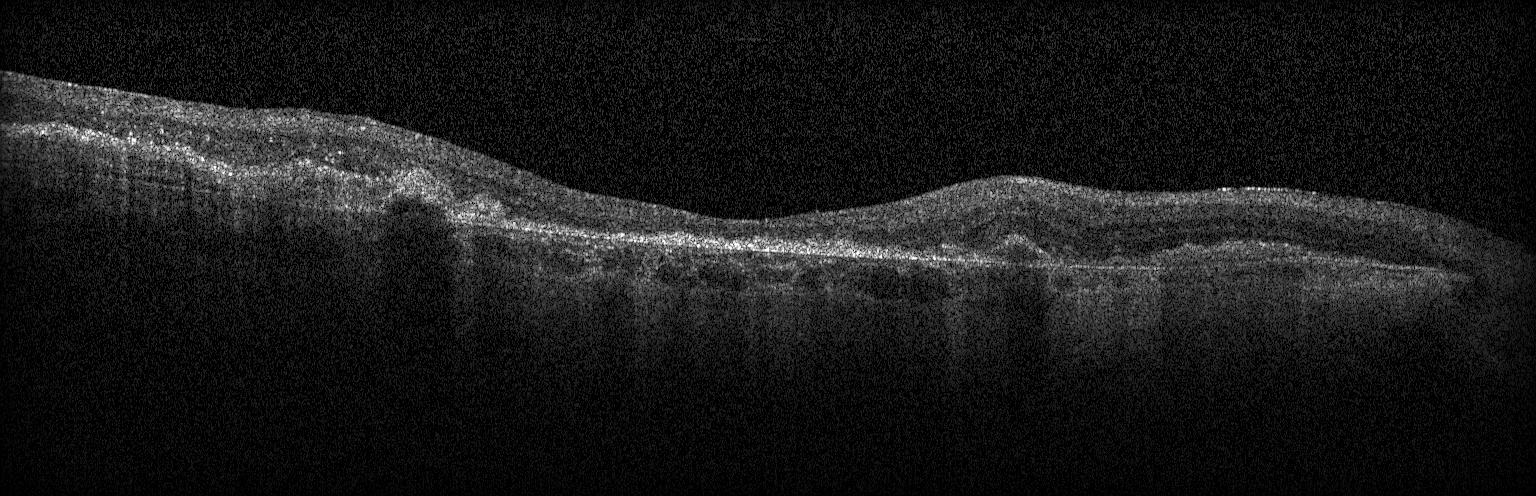

OCT B-scan. This B-scan demonstrates a choroidal neovascular membrane.